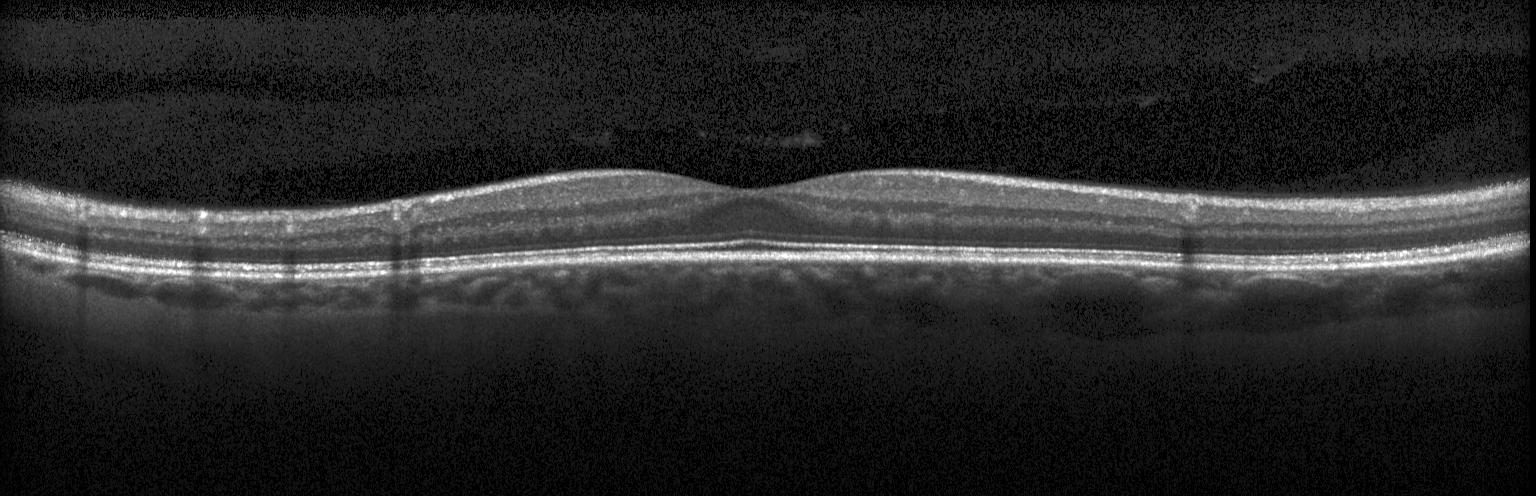 Retinal OCT B-scan, Heidelberg Spectralis, spectral-domain OCT. Macular OCT: no evidence of choroidal neovascularization, diabetic macular edema, or drusen.